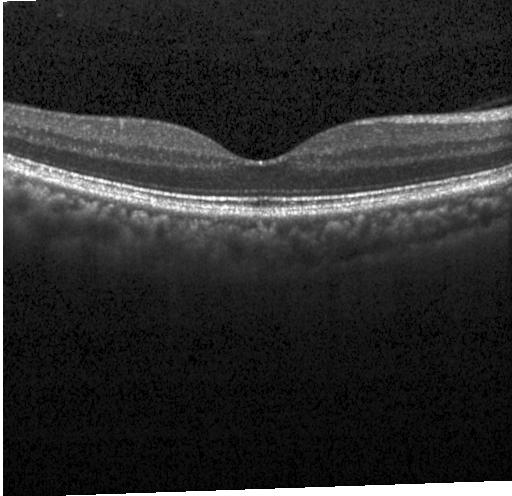

Spectral-domain optical coherence tomography; optical coherence tomography scan
Finding: no CNV, DME, or drusen.